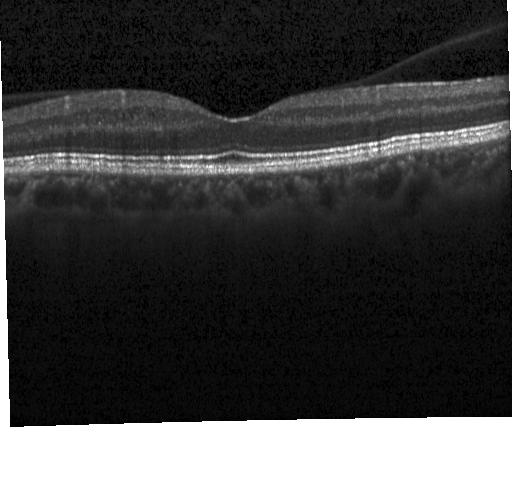
Heidelberg Spectralis. Horizontal scan through the fovea. Retinal OCT cross-section. Spectral-domain optical coherence tomography. No CNV, no DME, and no drusen.